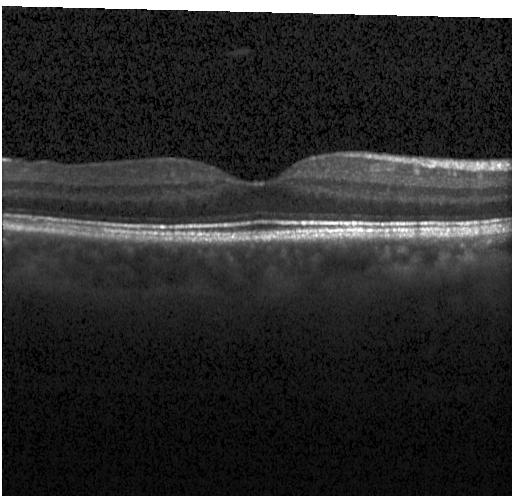

Dx: no choroidal neovascularization, diabetic macular edema, or drusen.